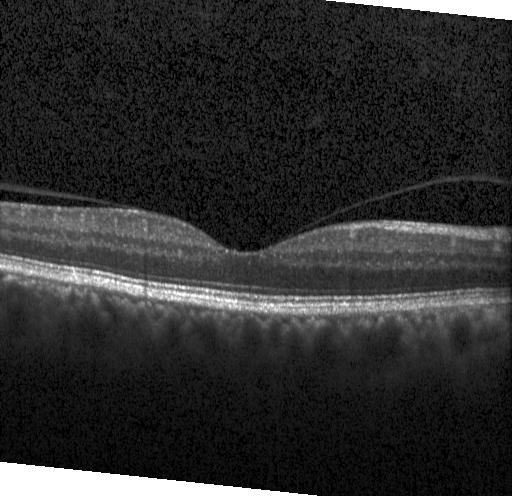

Fovea-centered; spectral-domain optical coherence tomography; retinal OCT B-scan; Heidelberg Spectralis OCT system
This B-scan demonstrates no evidence of choroidal neovascularization, diabetic macular edema, or drusen.